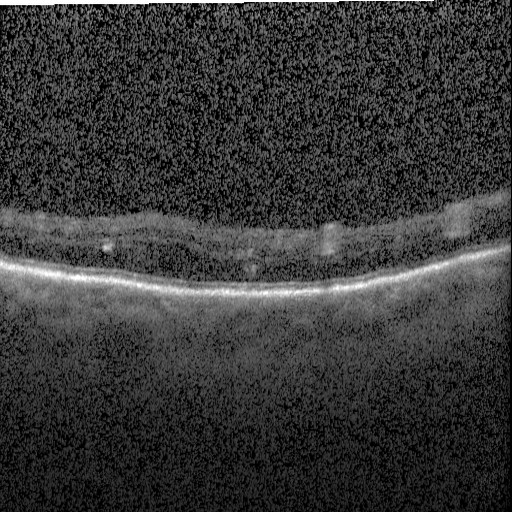

Retinal OCT cross-section; Heidelberg Spectralis OCT system; centered on the fovea — Finding: diabetic macular edema.